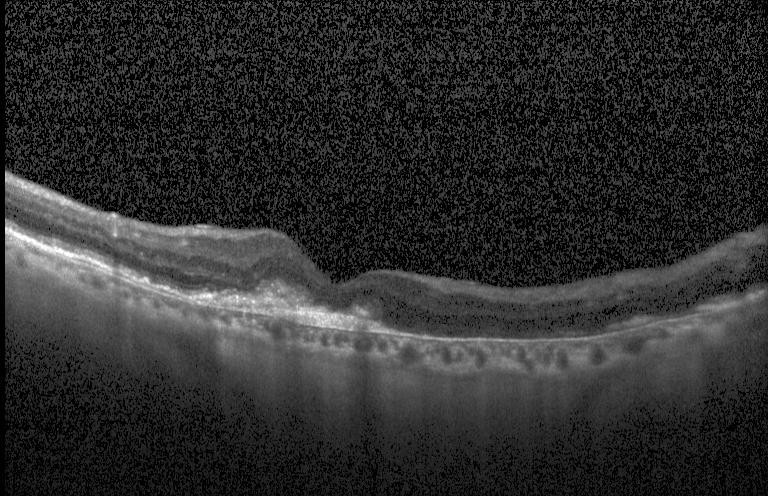 Optical coherence tomography B-scan. OCT finding: a choroidal neovascular membrane.